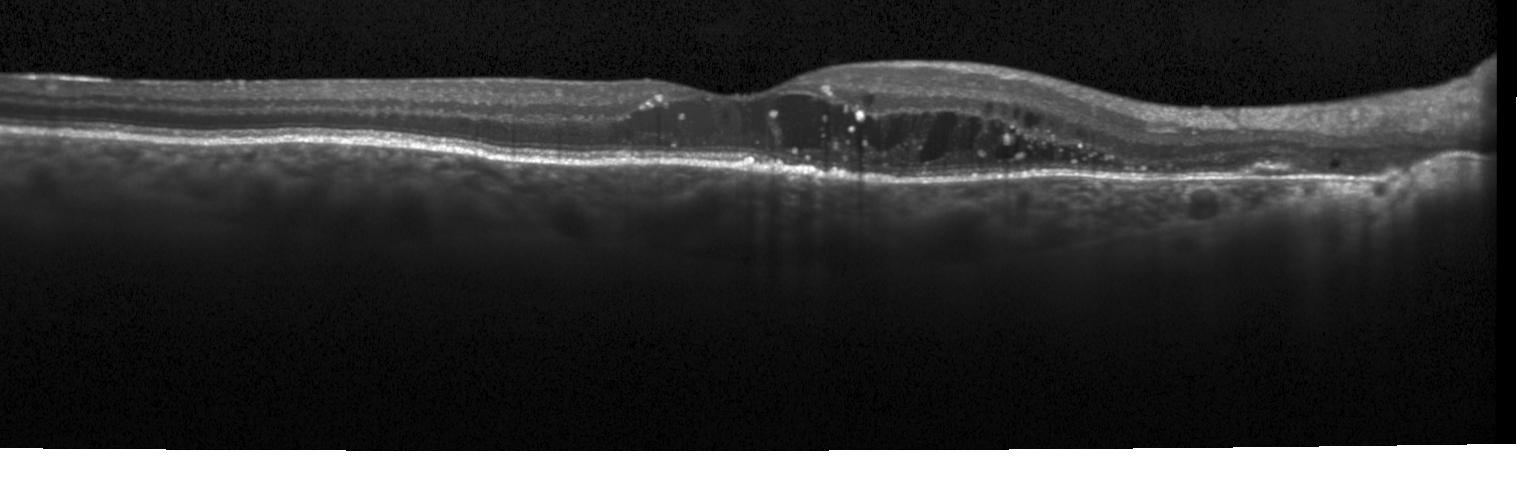
Dx: diabetic macular edema.